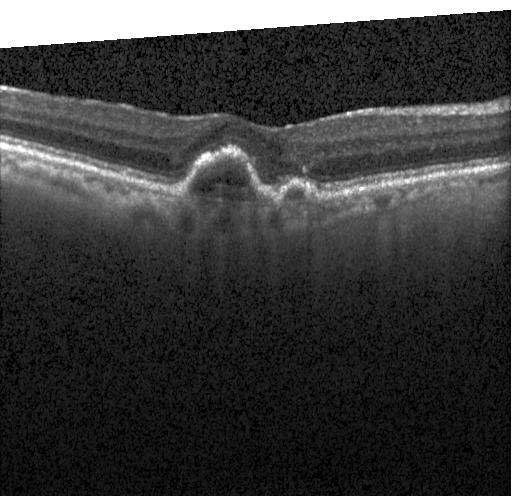 Retinal OCT cross-section, horizontal scan through the fovea.
The scan shows a choroidal neovascular membrane.